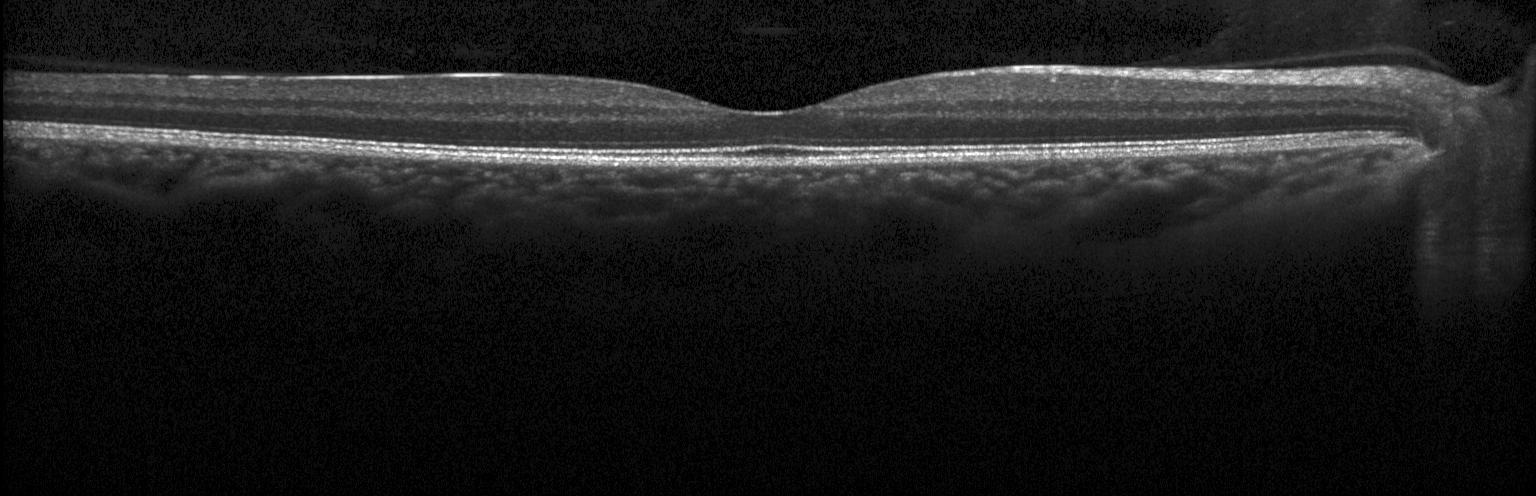
Macular OCT: no evidence of choroidal neovascularization, diabetic macular edema, or drusen.